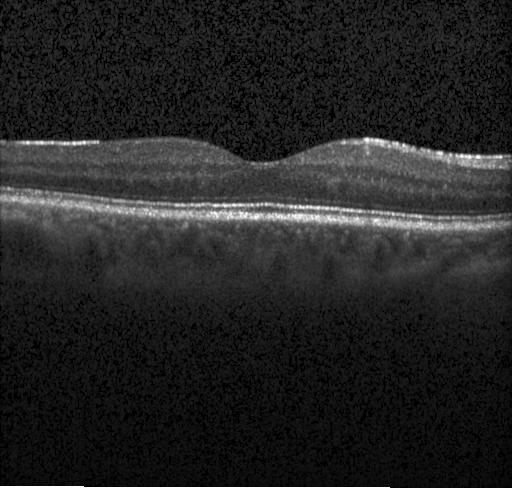 OCT scan showing no evidence of choroidal neovascularization, diabetic macular edema, or drusen.